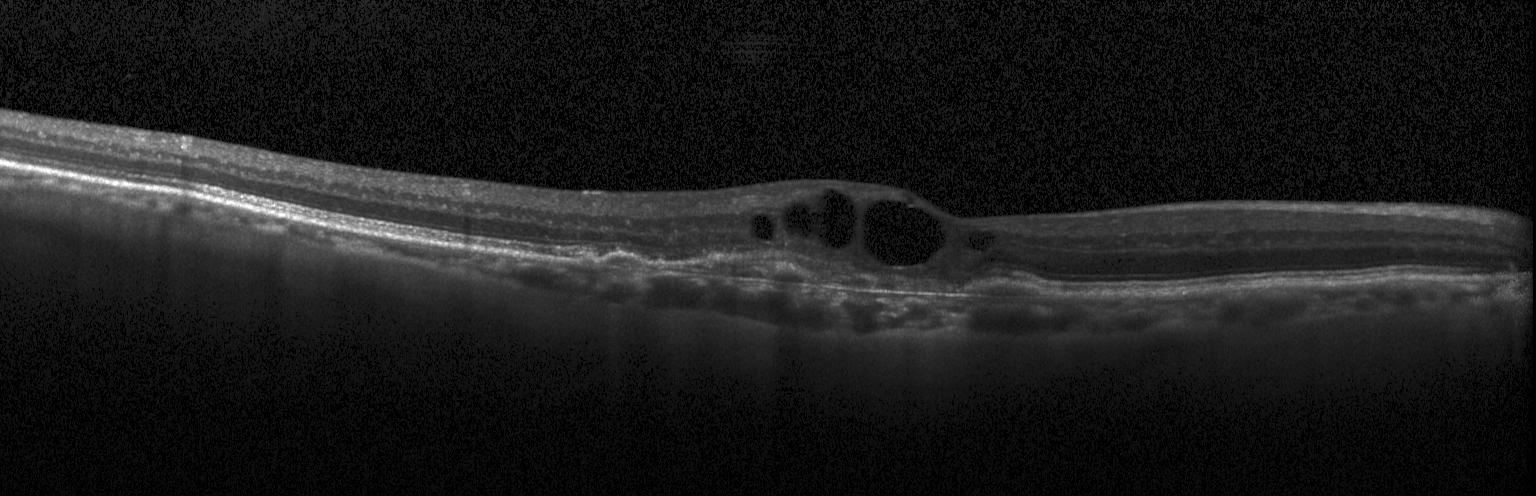

Acquired on a Heidelberg Spectralis · through the macula · retinal OCT cross-section.
A choroidal neovascular membrane.